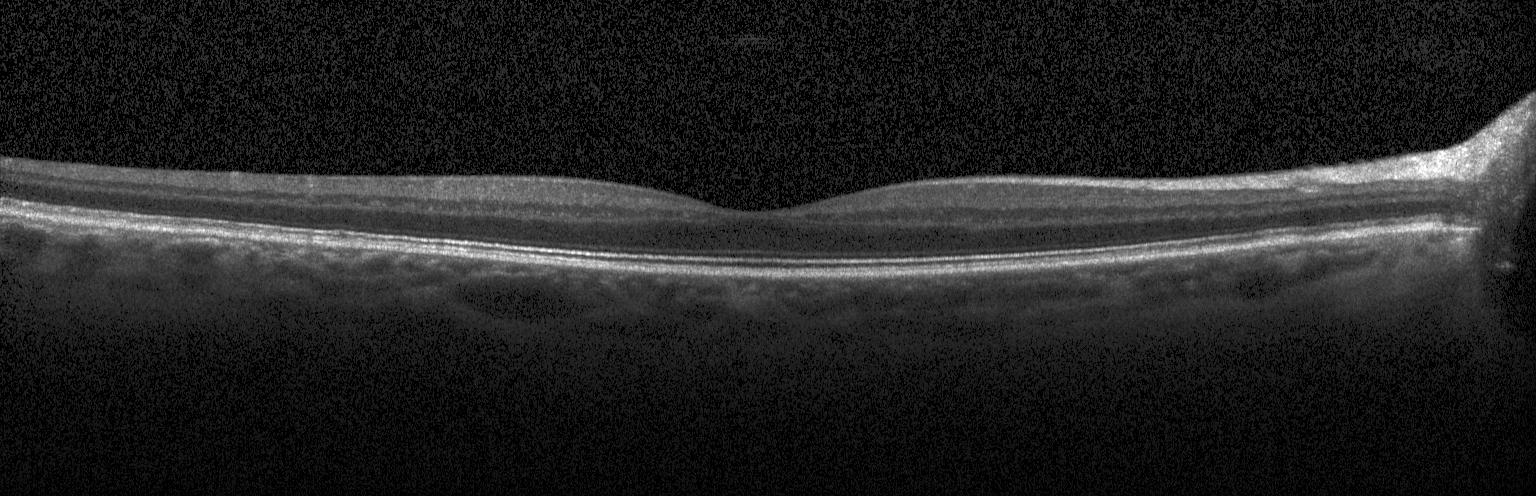 SD-OCT; retinal OCT cross-section.
Diagnosis: no evidence of CNV, DME, or drusen.